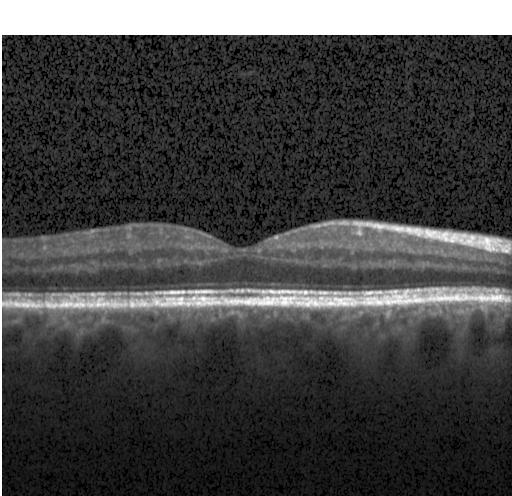 Diagnosis: no CNV, DME, or drusen.